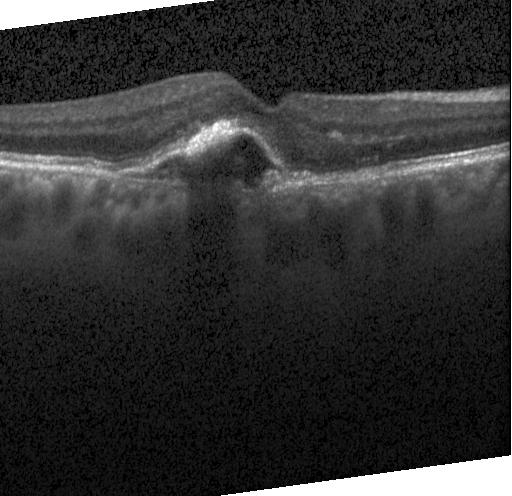
Retinal OCT cross-section
The scan shows CNV.